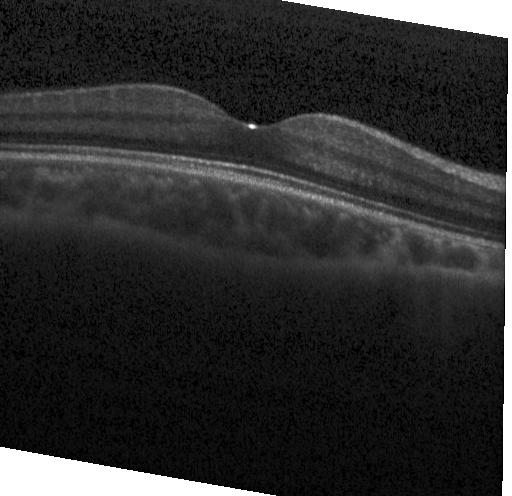 OCT line scan — Diagnosis: neither choroidal neovascularization, diabetic macular edema, nor drusen.